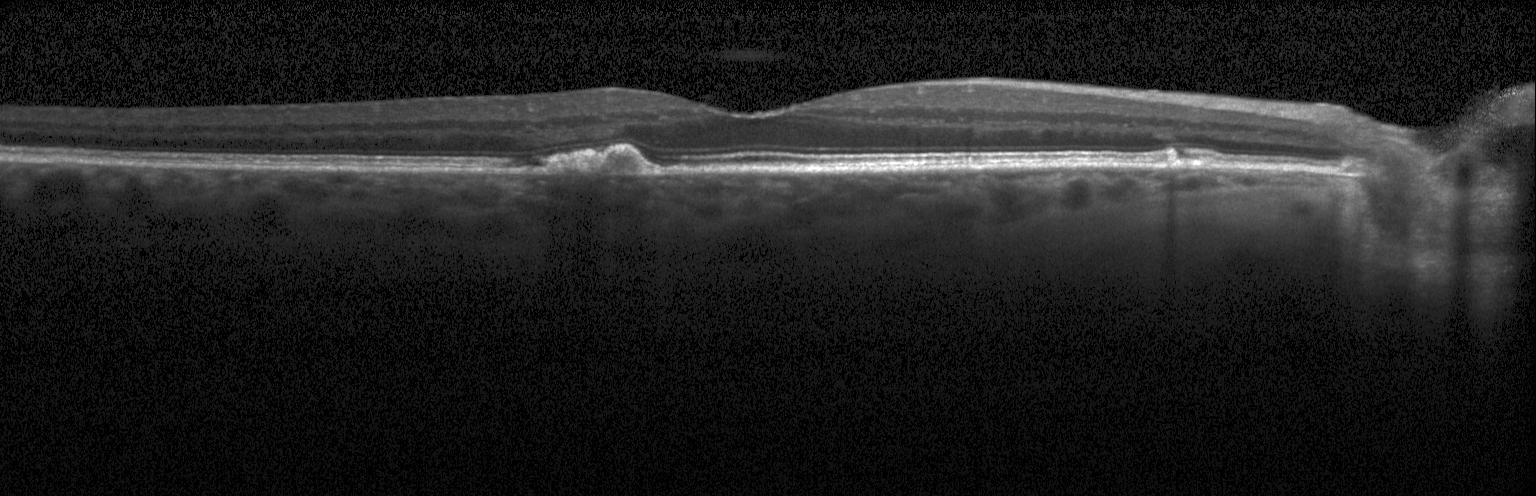

Diagnosis: a choroidal neovascular membrane.